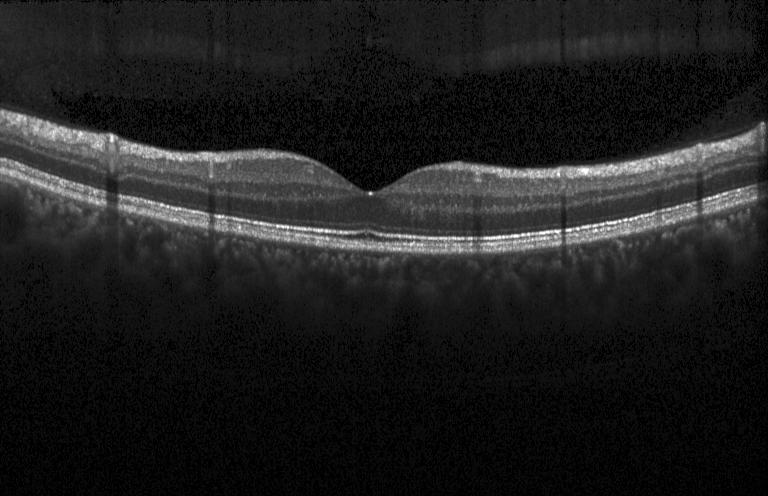

SD-OCT, retinal OCT cross-section — Diagnosis: no evidence of choroidal neovascularization, diabetic macular edema, or drusen.